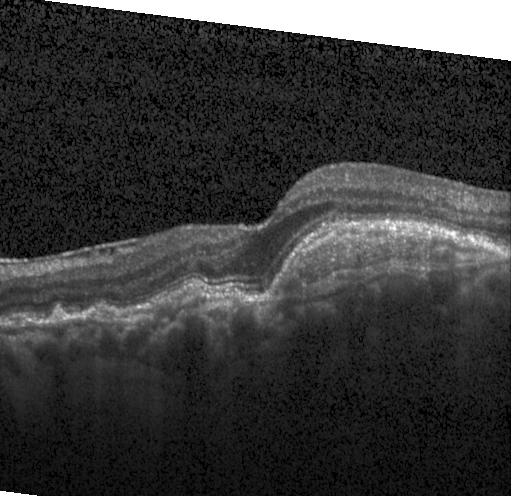

Optical coherence tomography B-scan; through the macula; spectral-domain optical coherence tomography. Choroidal neovascularization (CNV).